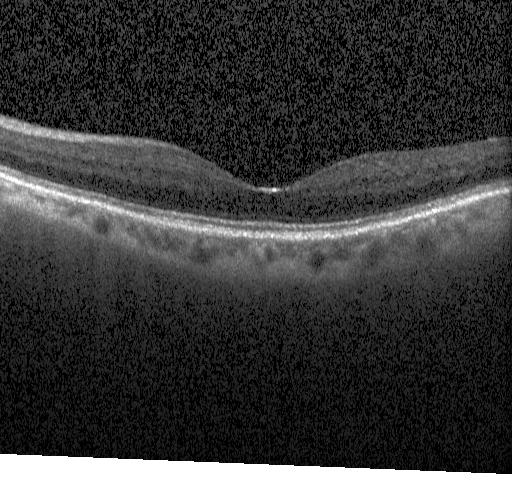

Fovea-centered. Retinal OCT B-scan. Macular OCT: neither CNV, DME, nor drusen.